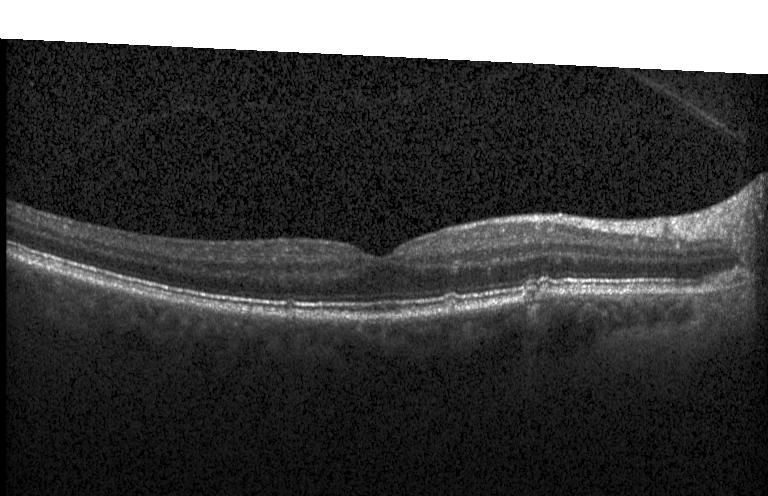
Through the macula · instrument: Heidelberg Spectralis · optical coherence tomography B-scan · spectral-domain OCT. Assessment: sub-RPE drusenoid deposits.